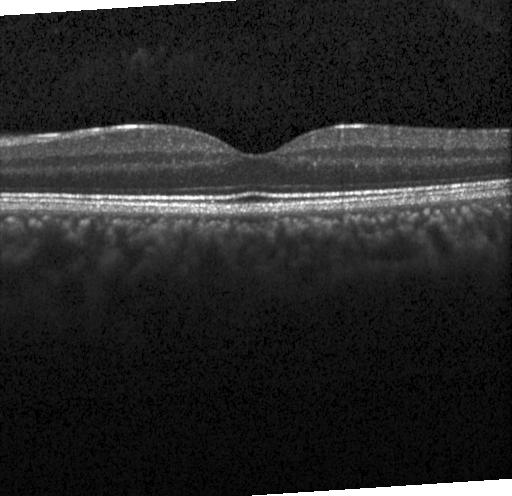

Dx: no choroidal neovascularization, no diabetic macular edema, and no drusen.